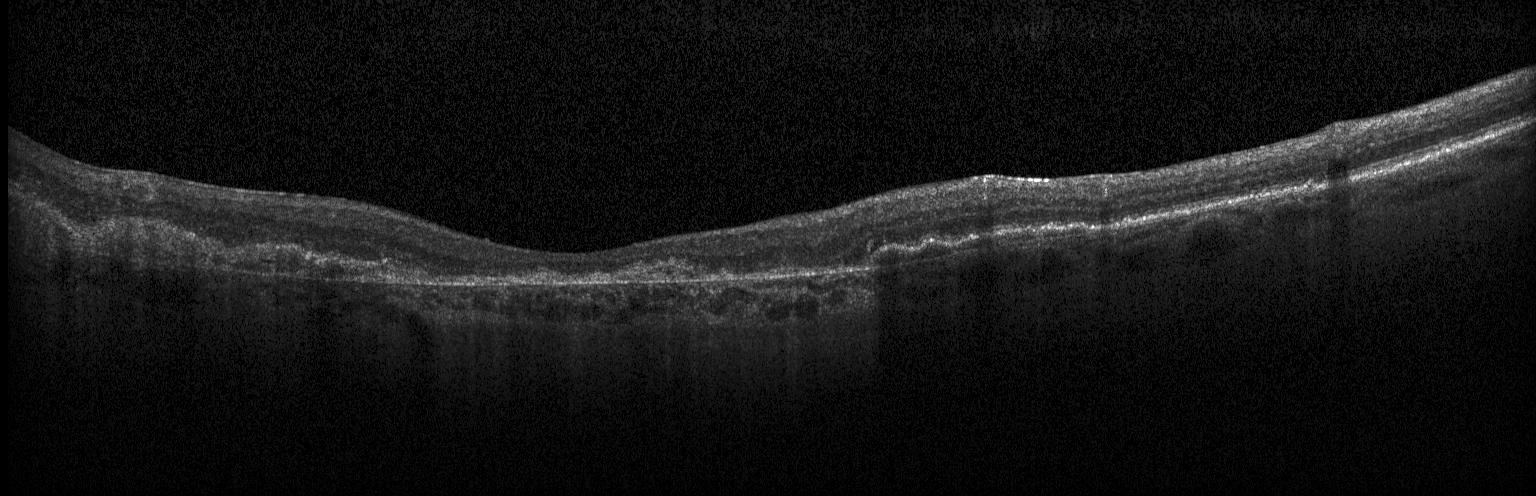

Retinal OCT cross-section showing choroidal neovascularization.